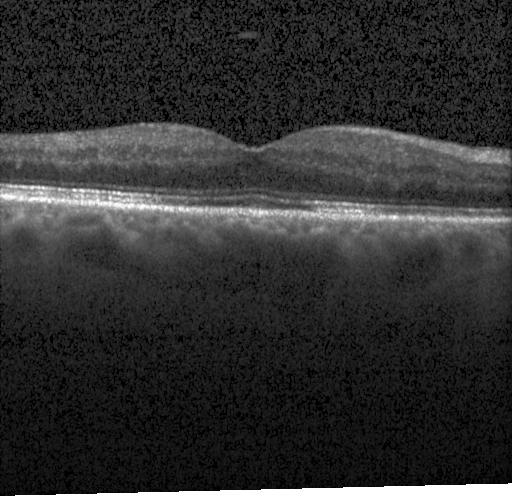 Heidelberg Spectralis, fovea-centered, optical coherence tomography B-scan, spectral-domain optical coherence tomography.
This B-scan demonstrates no CNV, DME, or drusen.